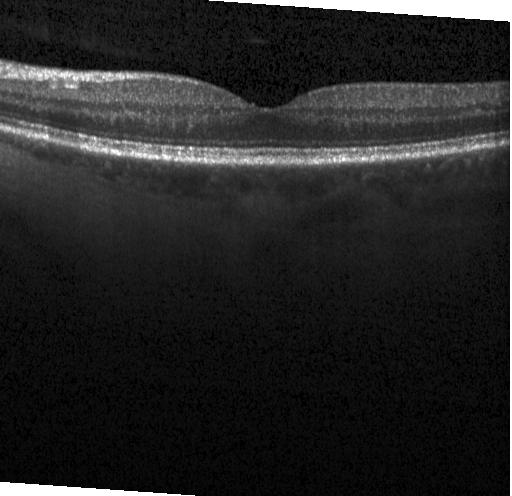
OCT finding: no CNV, no DME, and no drusen.